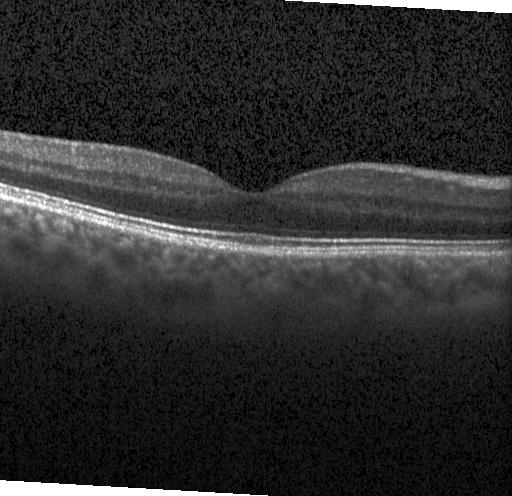

Spectral-domain optical coherence tomography; horizontal scan through the fovea; optical coherence tomography B-scan; acquired on a Heidelberg Spectralis.
Diagnosis: no choroidal neovascularization, diabetic macular edema, or drusen.